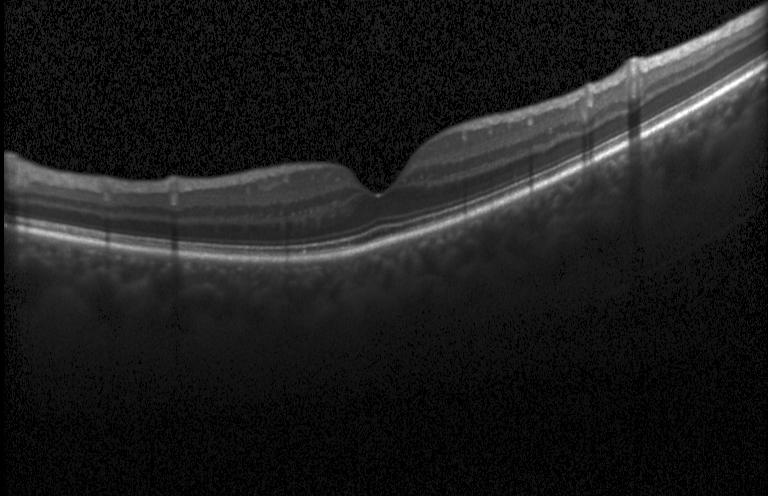

Diagnosis: neither choroidal neovascularization, diabetic macular edema, nor drusen.